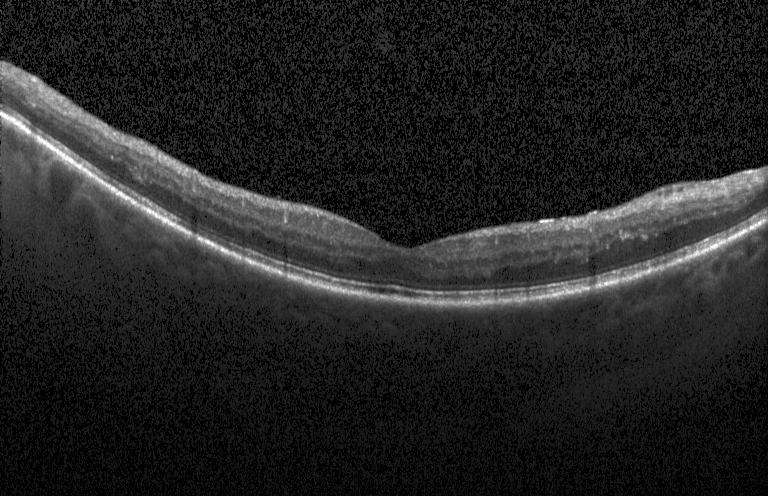

Finding: no choroidal neovascularization, diabetic macular edema, or drusen.